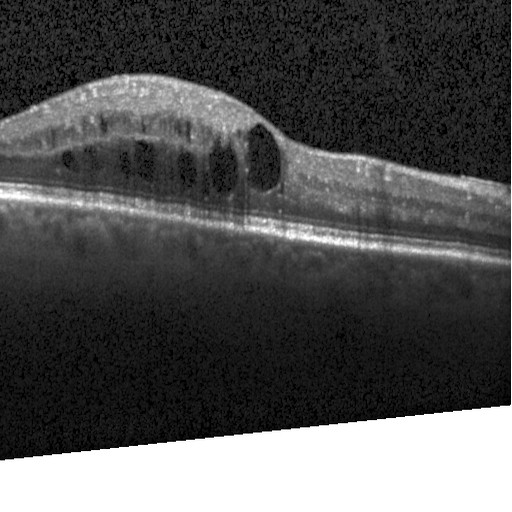 Optical coherence tomography B-scan
Assessment: DME.